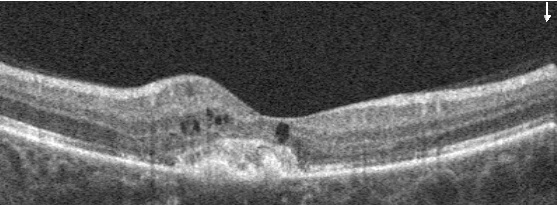

Optical coherence tomography scan · instrument: Optovue Avanti RTVue XR. Finding: age-related macular degeneration.